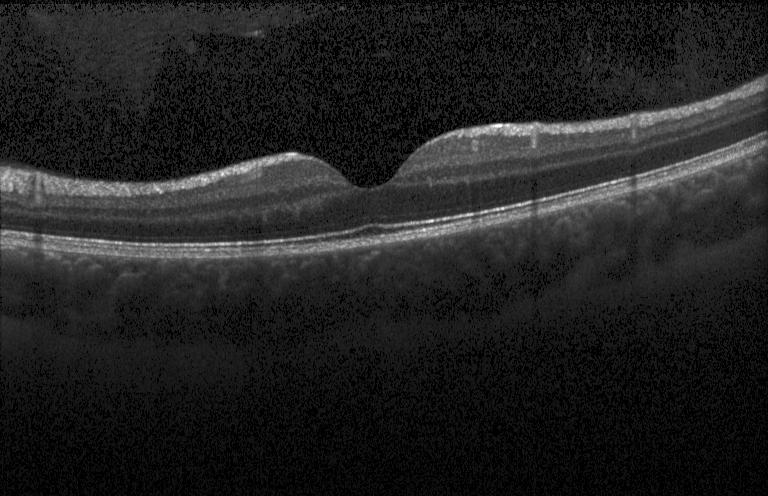

Macular OCT: no choroidal neovascularization, diabetic macular edema, or drusen.